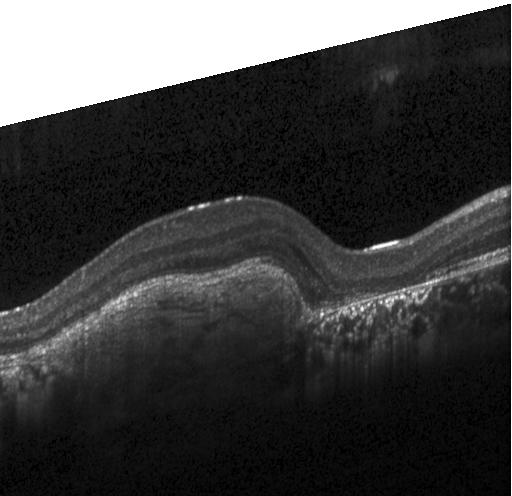 Dx: choroidal neovascularization.